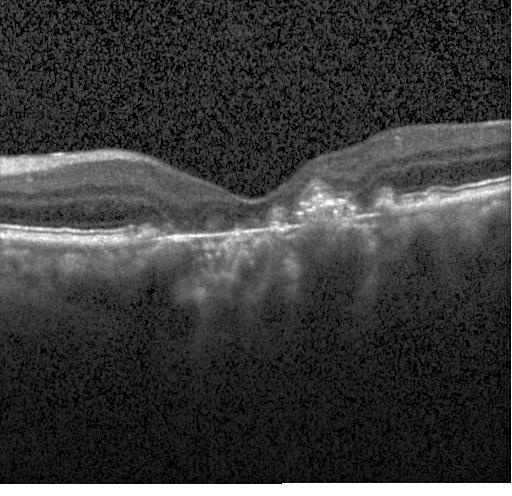
OCT B-scan, Heidelberg Spectralis, centered on the fovea, SD-OCT.
This B-scan demonstrates choroidal neovascularization.